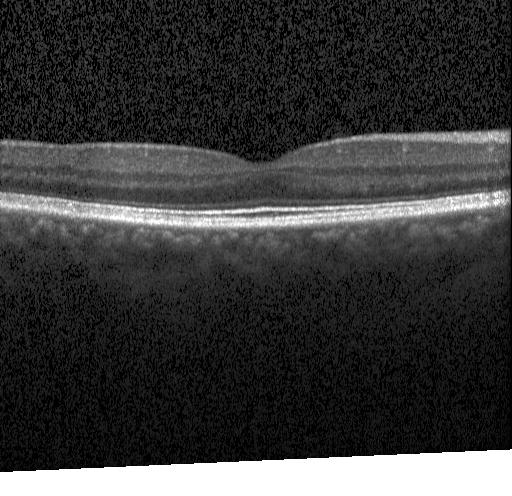

Assessment: no evidence of choroidal neovascularization, diabetic macular edema, or drusen.